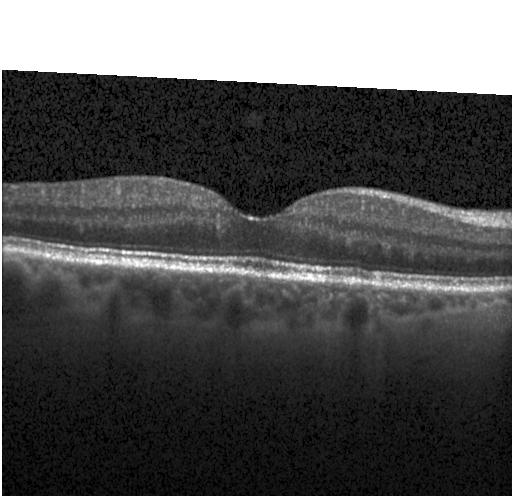 Heidelberg Spectralis OCT system. Retinal OCT cross-section — Impression: no choroidal neovascularization, diabetic macular edema, or drusen.